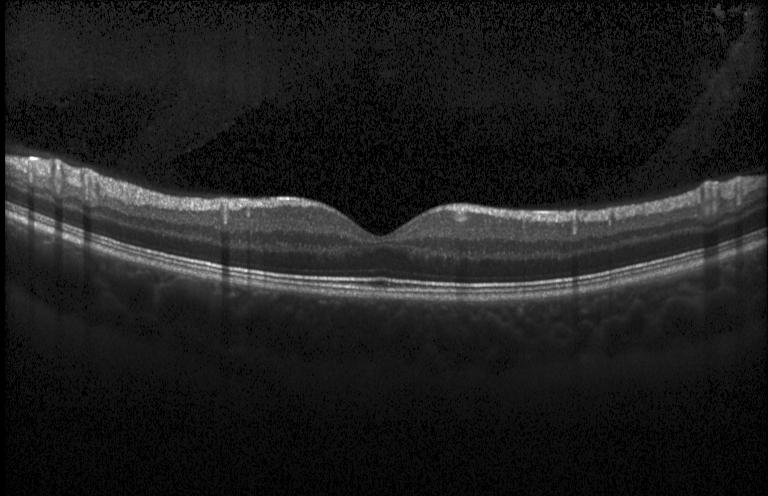 Retinal OCT cross-section · fovea-centered — Diagnosis: no evidence of choroidal neovascularization, diabetic macular edema, or drusen.